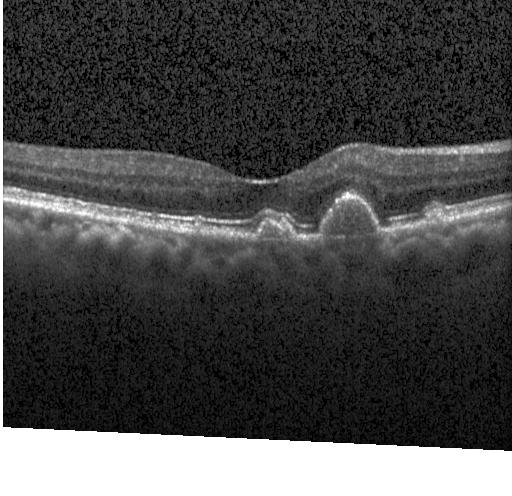 Impression: drusen.